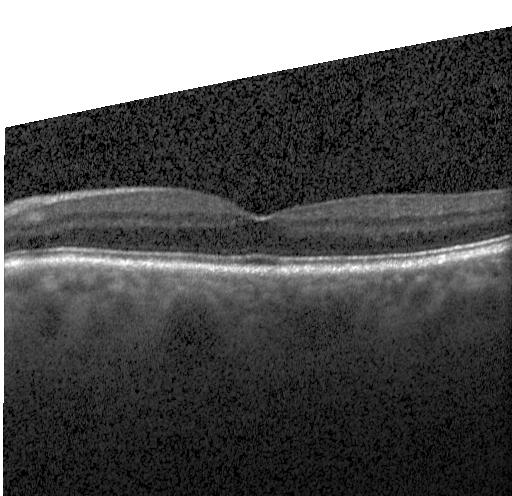

No CNV, DME, or drusen.